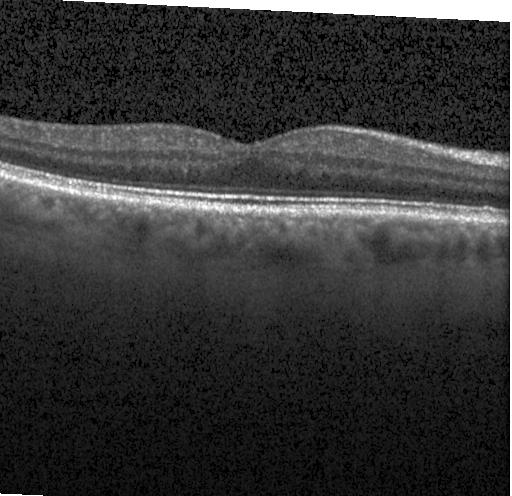
No choroidal neovascularization, diabetic macular edema, or drusen.